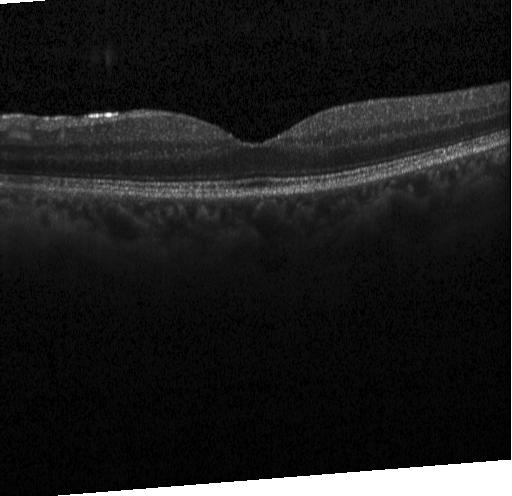

Centered on the fovea. Optical coherence tomography scan. SD-OCT — Macular OCT: no choroidal neovascularization, diabetic macular edema, or drusen.